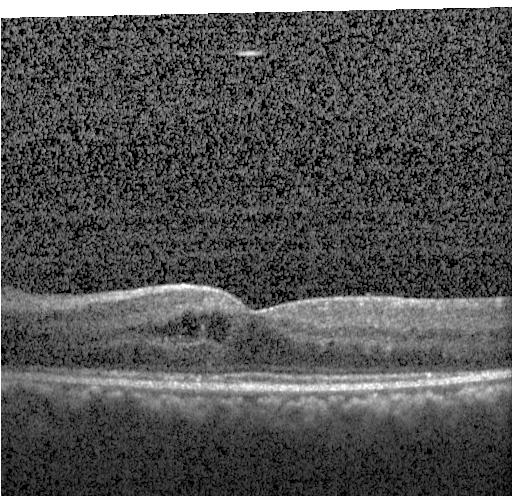

Through the macula. Acquired on a Heidelberg Spectralis. Optical coherence tomography B-scan — Diagnosis: diabetic macular edema (DME).